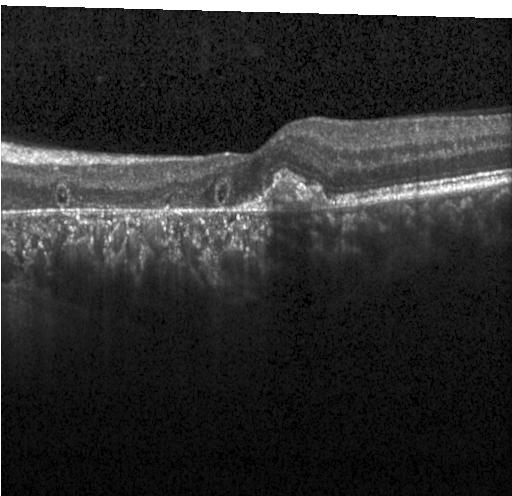 Centered on the fovea; spectral-domain OCT; OCT line scan; Heidelberg Spectralis OCT system — Assessment: a choroidal neovascular membrane.